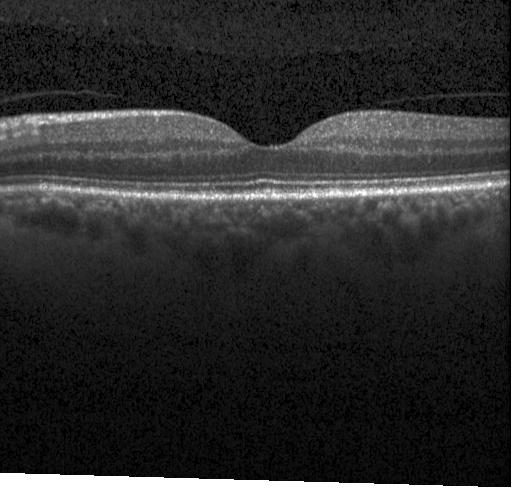

Optical coherence tomography scan. Heidelberg Spectralis OCT system — The scan shows no CNV, DME, or drusen.